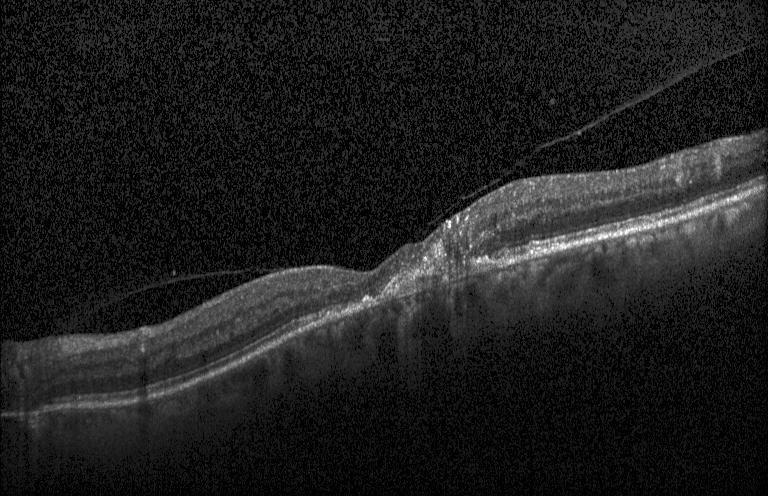

Heidelberg Spectralis OCT system · SD-OCT · optical coherence tomography scan · horizontal scan through the fovea.
Impression: CNV.